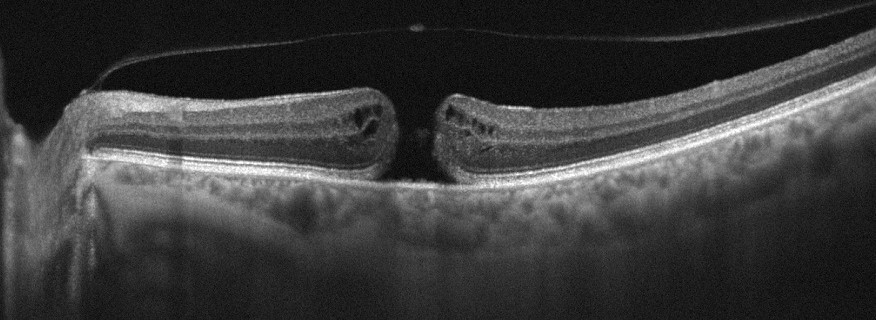
Diagnosis: vitreomacular interface disease.